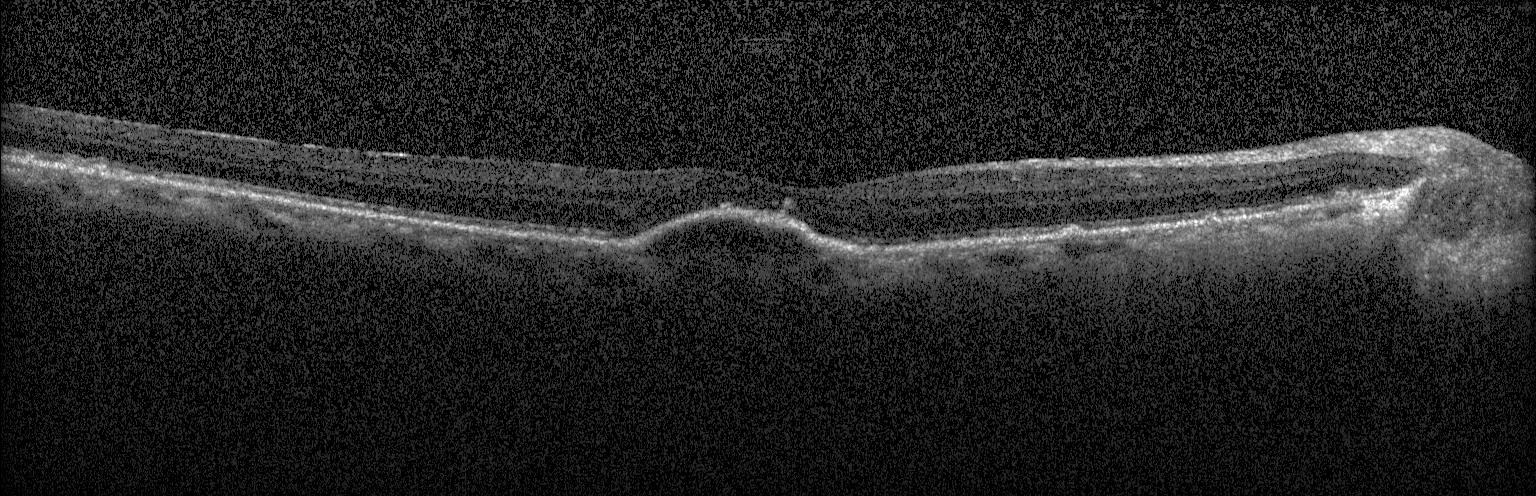

SD-OCT · through the macula · Heidelberg Spectralis · optical coherence tomography scan.
OCT finding: CNV.